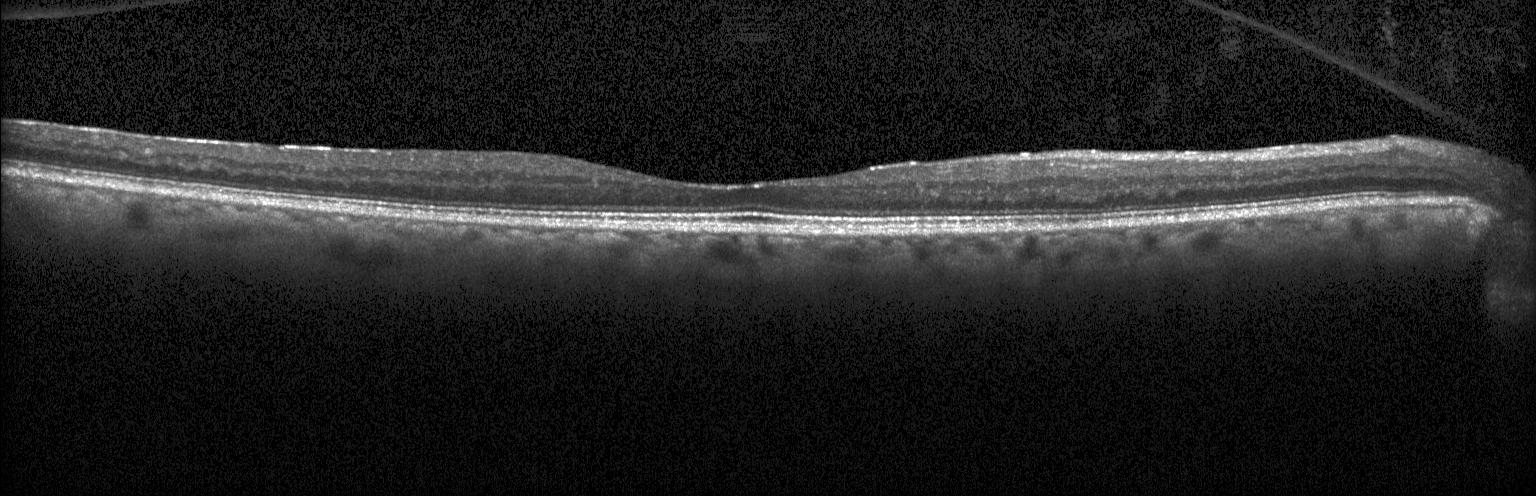 OCT line scan.
Finding: neither choroidal neovascularization, diabetic macular edema, nor drusen.